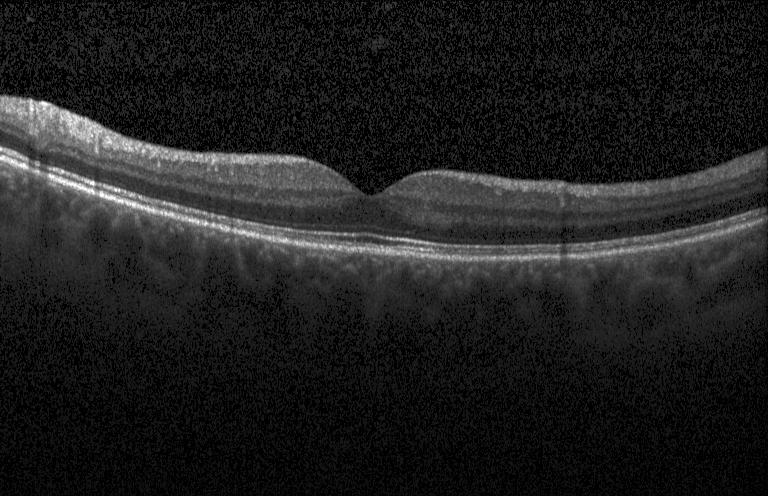 Spectral-domain OCT B-scan: no choroidal neovascularization, no diabetic macular edema, and no drusen.